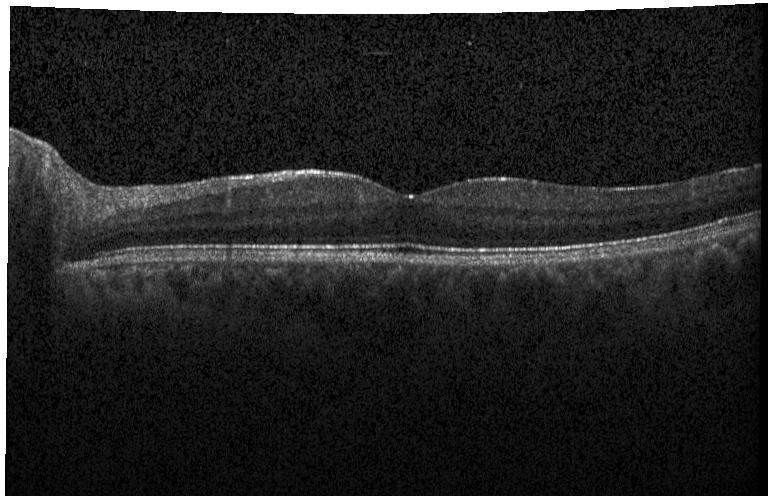

Finding: no CNV, no DME, and no drusen.